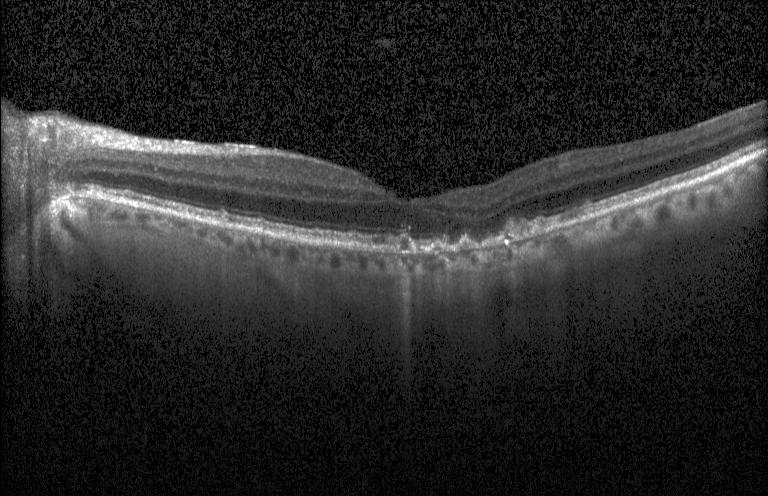

Centered on the fovea. Instrument: Heidelberg Spectralis. Retinal OCT cross-section. Spectral-domain OCT. The scan shows sub-RPE drusenoid deposits.